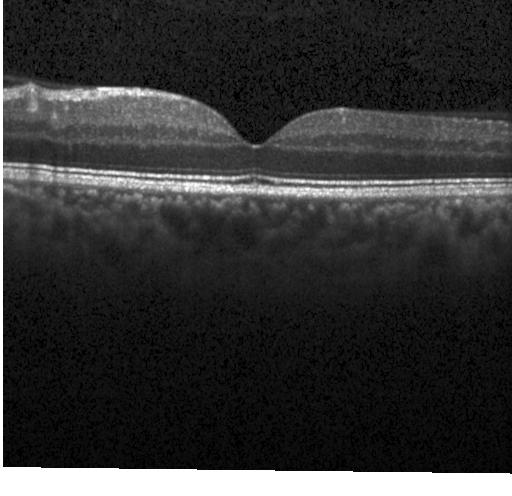

Acquired on a Heidelberg Spectralis; SD-OCT; fovea-centered; OCT line scan.
Finding: no evidence of CNV, DME, or drusen.